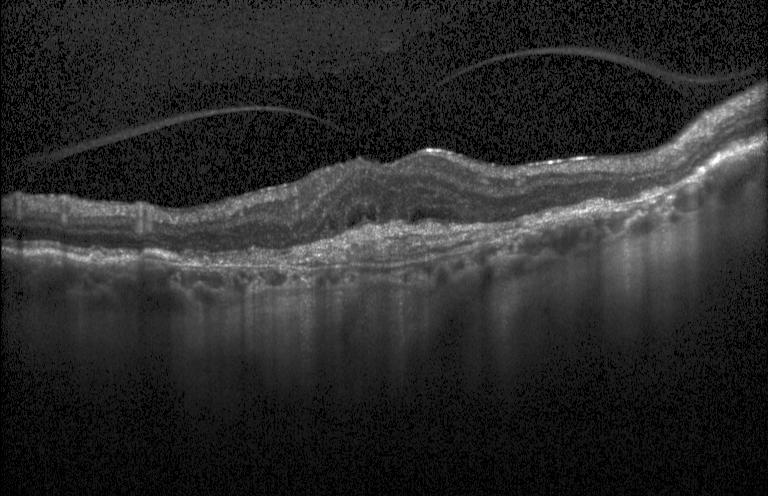

OCT B-scan showing CNV.